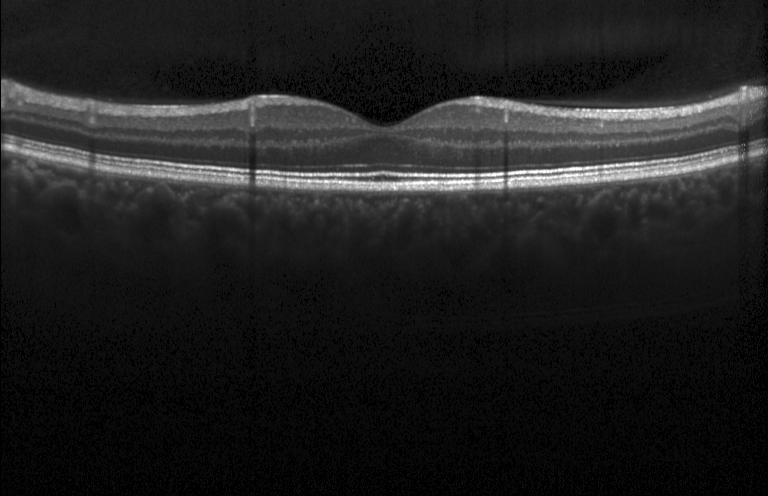

Fovea-centered; spectral-domain OCT; retinal OCT cross-section.
Finding: no evidence of CNV, DME, or drusen.